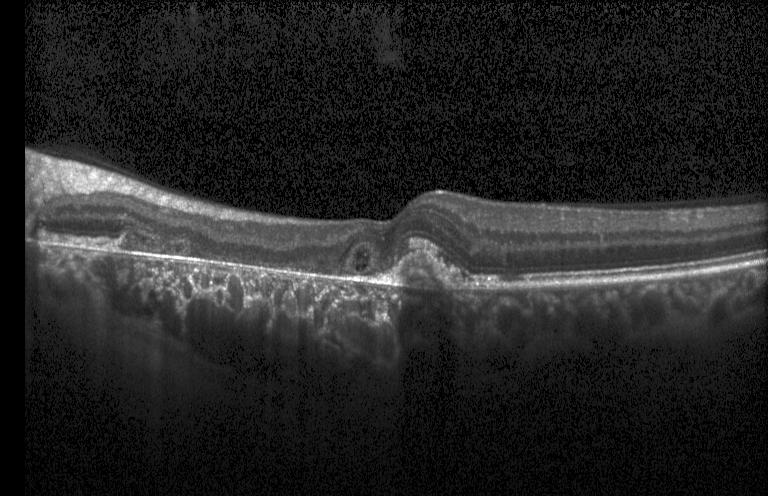
OCT line scan; Heidelberg Spectralis OCT system; SD-OCT. Dx: a choroidal neovascular membrane.